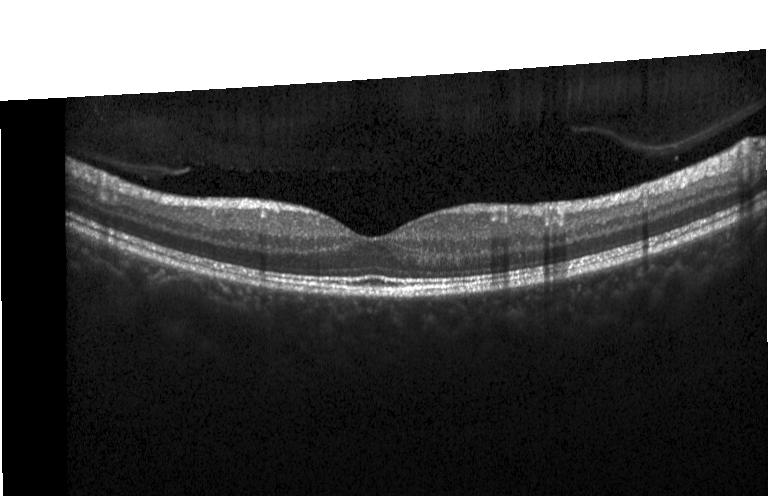
Finding: no evidence of choroidal neovascularization, diabetic macular edema, or drusen.